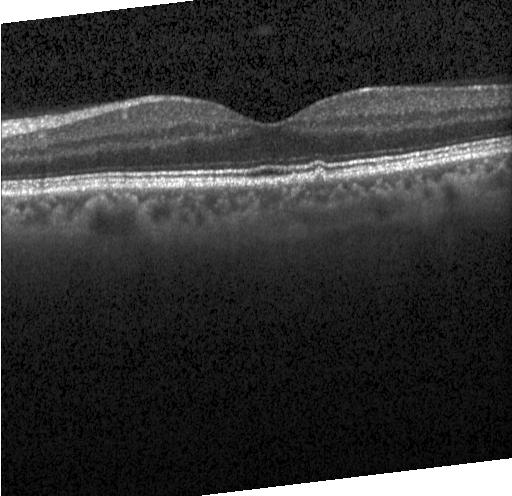

Macular scan, retinal OCT cross-section.
Dx: drusen.